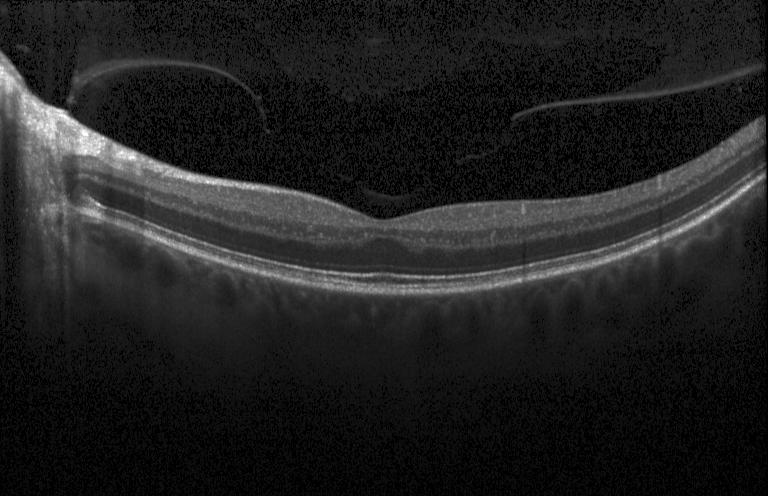 Diagnosis: no CNV, DME, or drusen.